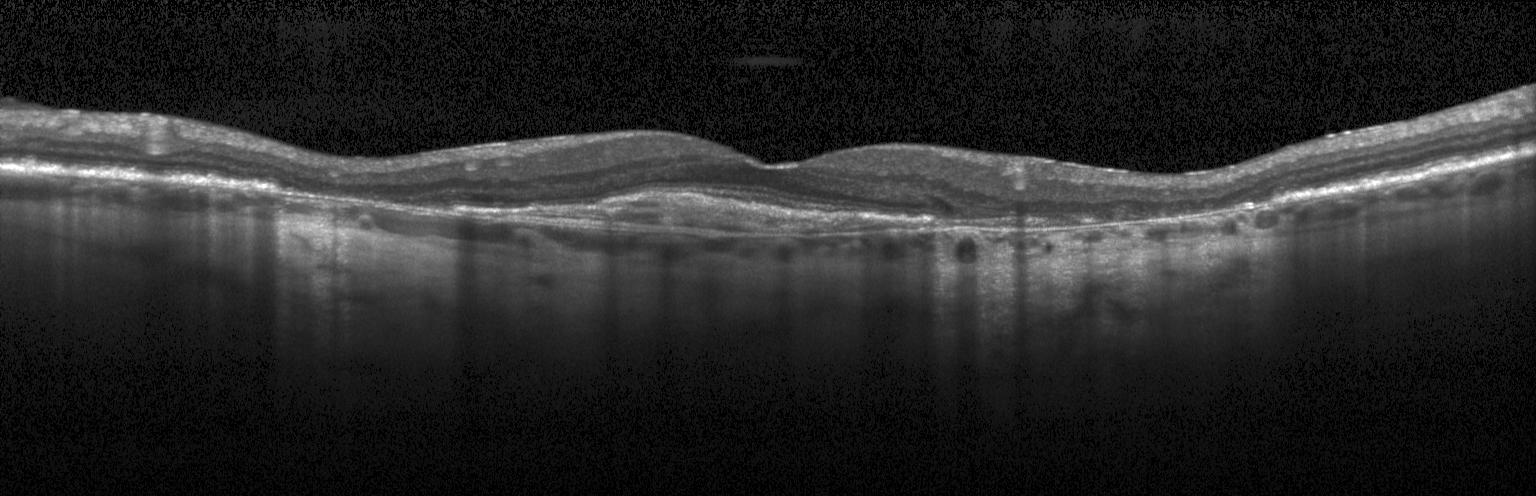 Retinal OCT cross-section, Heidelberg Spectralis OCT system
Diagnosis: choroidal neovascularization.